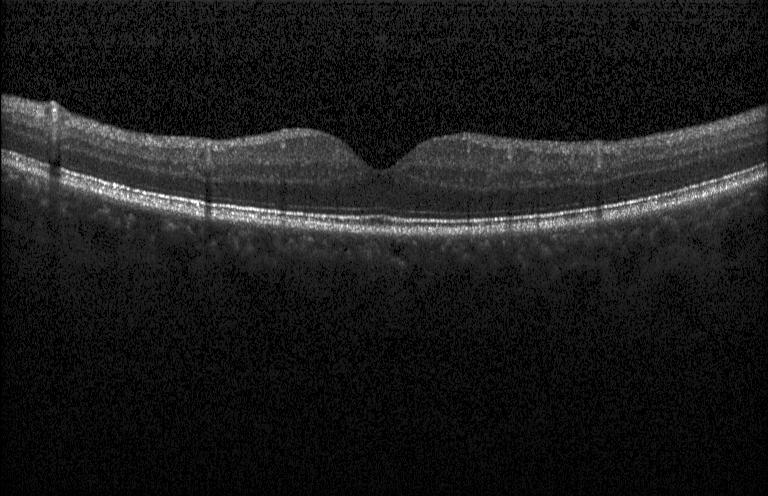
The scan shows no choroidal neovascularization, no diabetic macular edema, and no drusen.